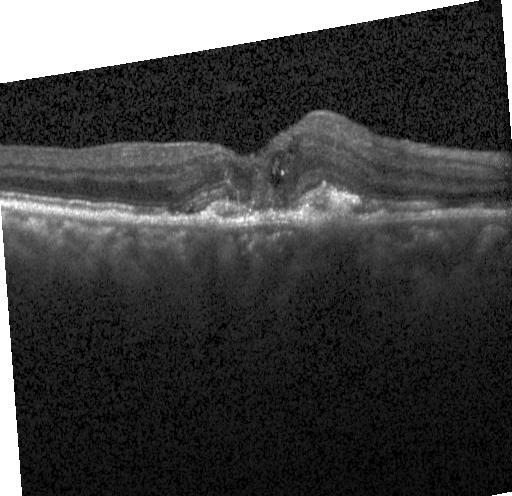 SD-OCT. Optical coherence tomography scan. Heidelberg Spectralis OCT system. Macular scan
Choroidal neovascularization (CNV).